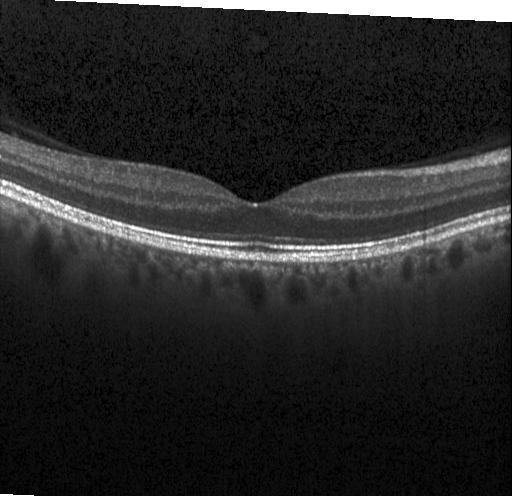

Macular OCT: no choroidal neovascularization, diabetic macular edema, or drusen.